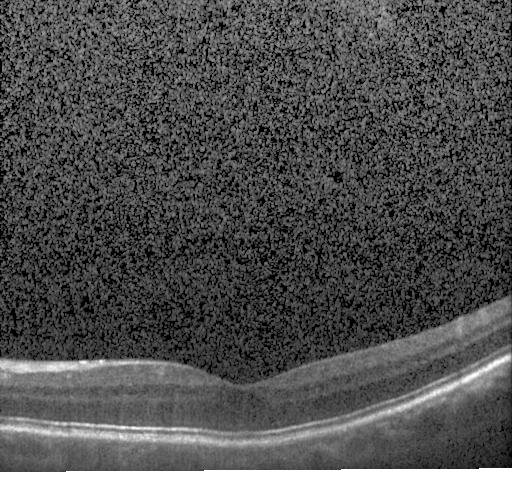 Retinal OCT cross-section showing neither choroidal neovascularization, diabetic macular edema, nor drusen.